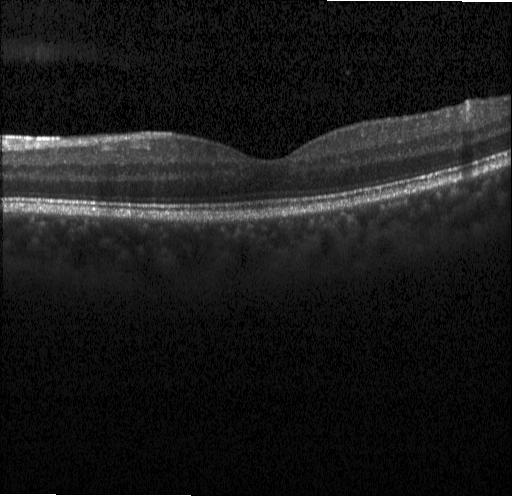

Acquired on a Heidelberg Spectralis; horizontal scan through the fovea; OCT line scan; SD-OCT
Assessment: no evidence of CNV, DME, or drusen.